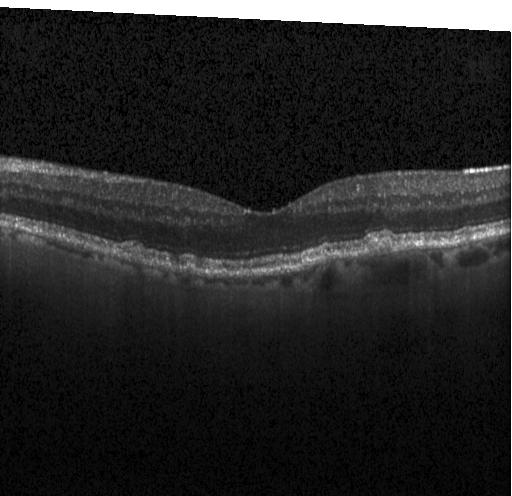

Spectral-domain OCT. Retinal OCT B-scan — Assessment: drusen.